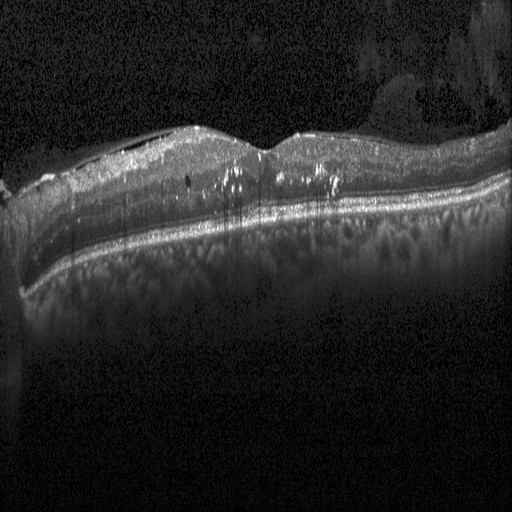
Finding: diabetic macular edema.